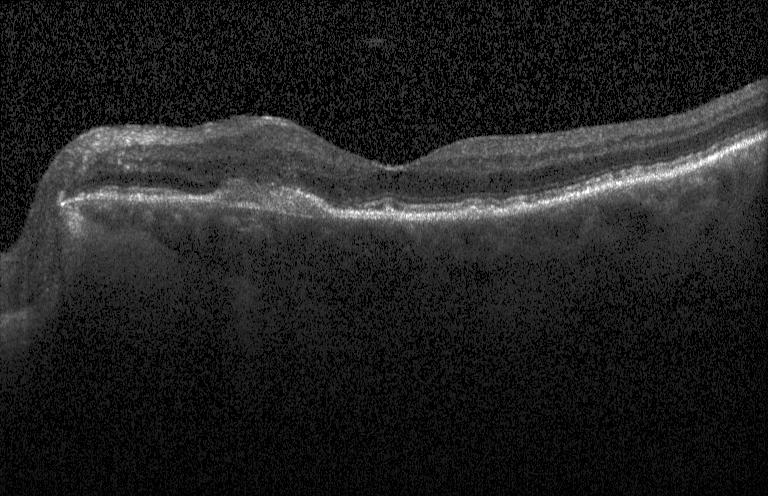 Macular scan · SD-OCT · retinal OCT B-scan.
The scan shows a choroidal neovascular membrane.